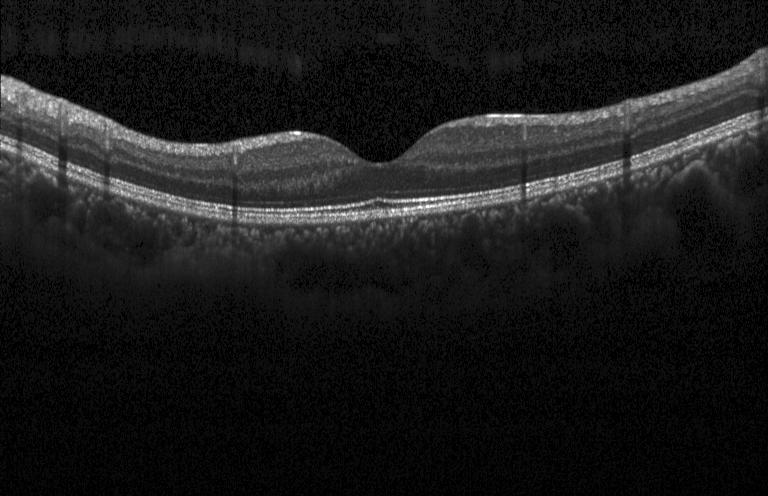
This B-scan demonstrates no choroidal neovascularization, no diabetic macular edema, and no drusen.